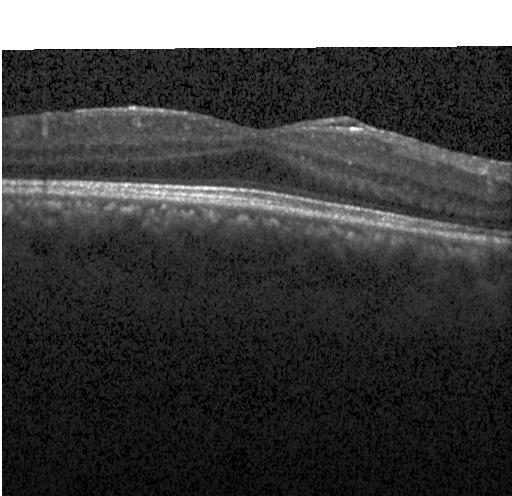
Spectral-domain optical coherence tomography; acquired on a Heidelberg Spectralis; retinal OCT B-scan; horizontal scan through the fovea. Finding: neither CNV, DME, nor drusen.